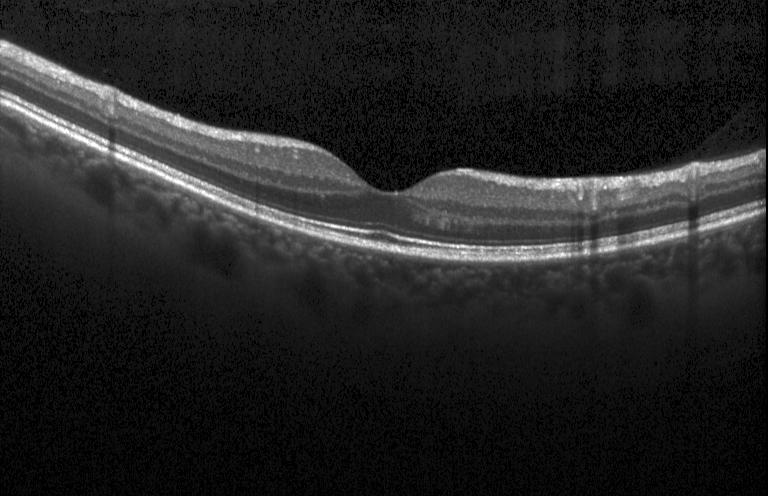
Optical coherence tomography B-scan.
Finding: no choroidal neovascularization, diabetic macular edema, or drusen.